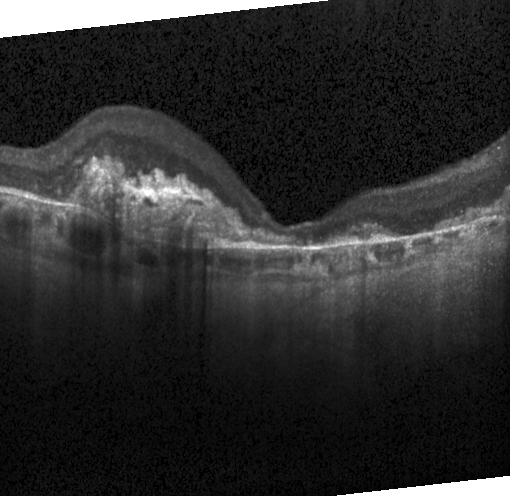

Retinal OCT B-scan · spectral-domain optical coherence tomography · macular scan — The scan shows choroidal neovascularization.